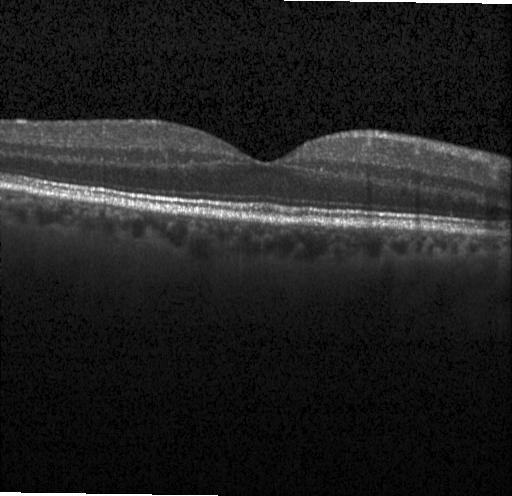 Acquired on a Heidelberg Spectralis · spectral-domain optical coherence tomography · retinal OCT cross-section · centered on the fovea
Diagnosis: neither choroidal neovascularization, diabetic macular edema, nor drusen.